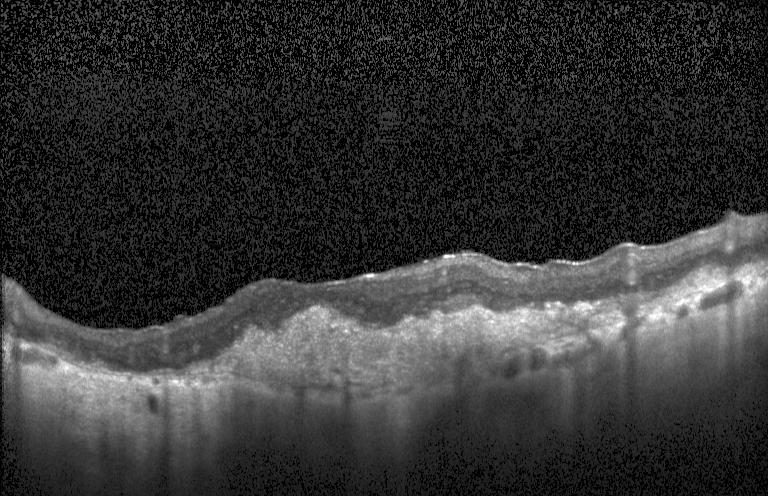
OCT scan showing choroidal neovascularization.